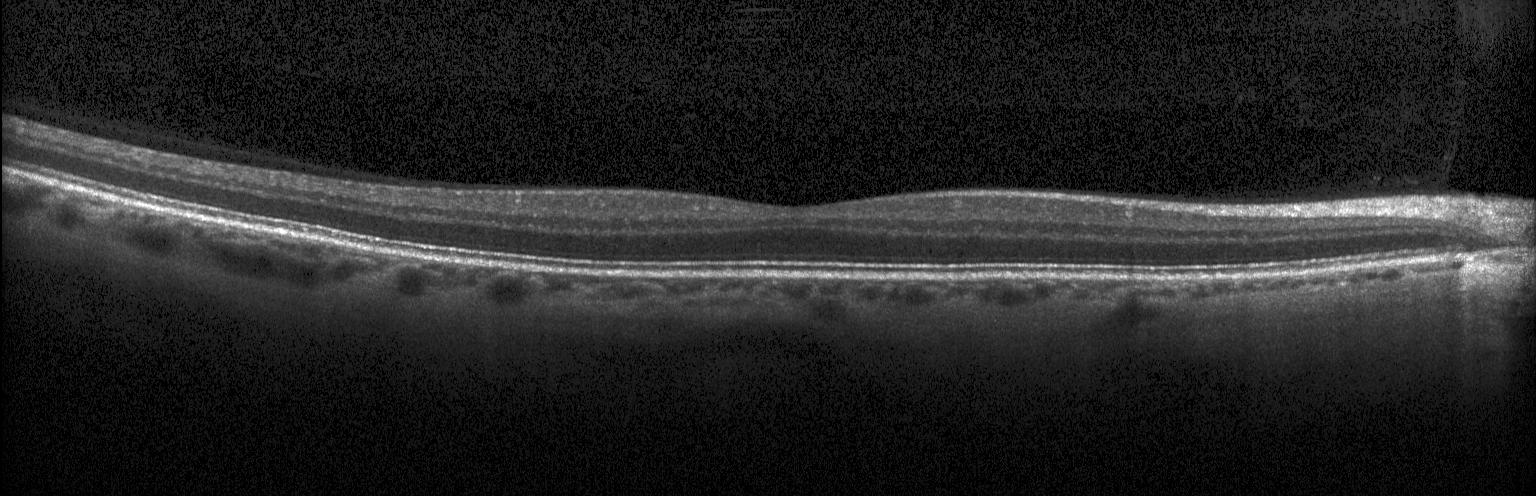
Optical coherence tomography B-scan
Assessment: no choroidal neovascularization, diabetic macular edema, or drusen.